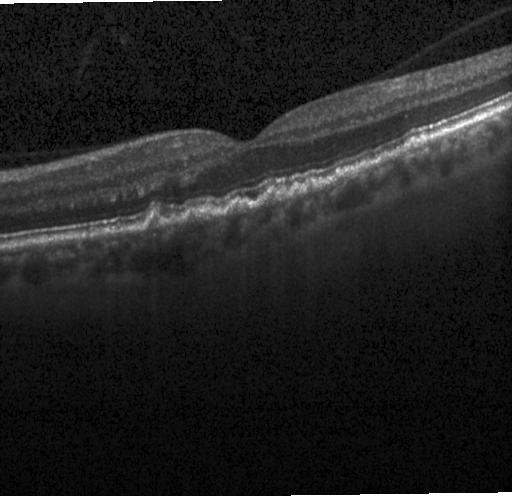
SD-OCT; retinal OCT B-scan; Heidelberg Spectralis OCT system; through the macula
This B-scan demonstrates multiple drusen.